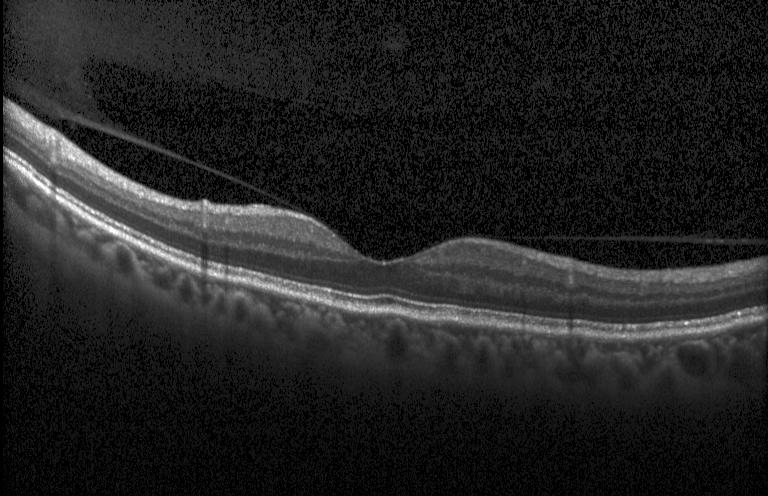 Optical coherence tomography scan; horizontal scan through the fovea
Assessment: no evidence of CNV, DME, or drusen.